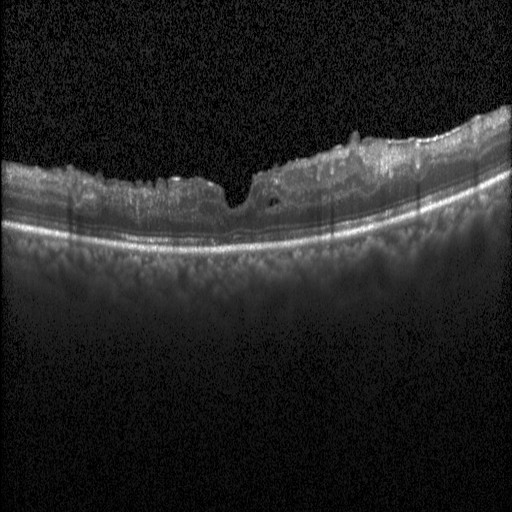
Optical coherence tomography scan; acquired on a Heidelberg Spectralis. Diagnosis: DME.